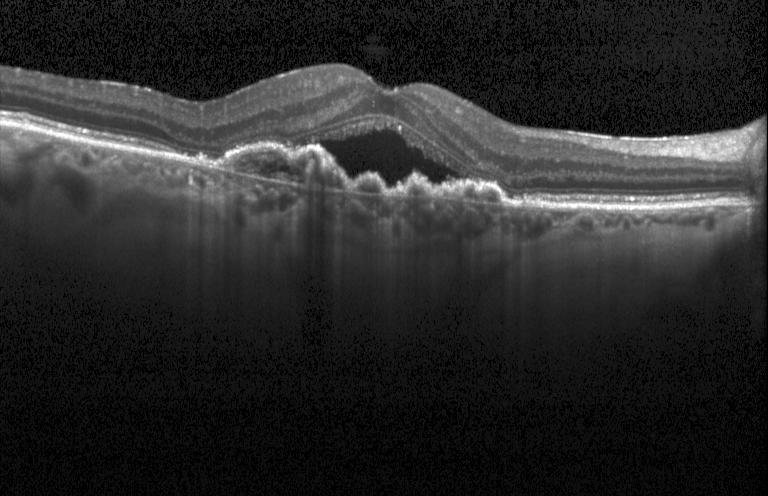 Impression: choroidal neovascularization.